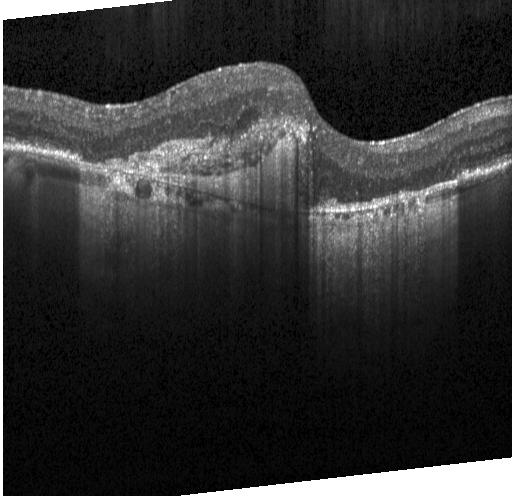
OCT scan showing a choroidal neovascular membrane.